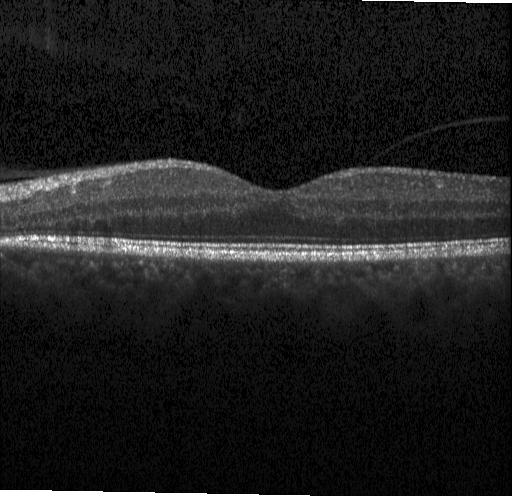 Spectral-domain OCT, OCT line scan, acquired on a Heidelberg Spectralis, centered on the fovea
The scan shows no evidence of choroidal neovascularization, diabetic macular edema, or drusen.